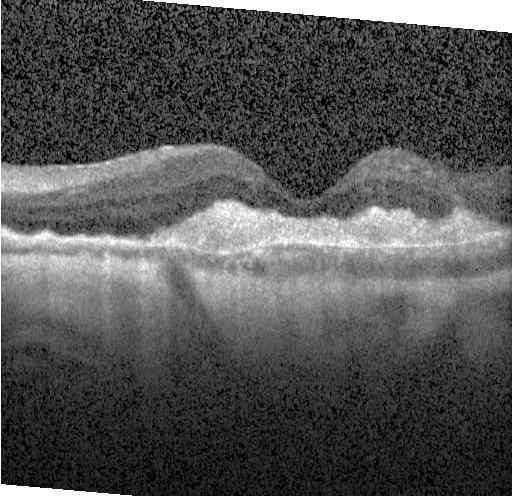
Optical coherence tomography scan — The scan shows CNV.